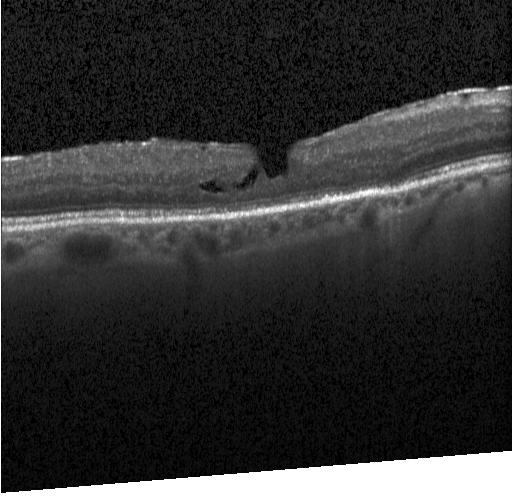
Impression: DME.